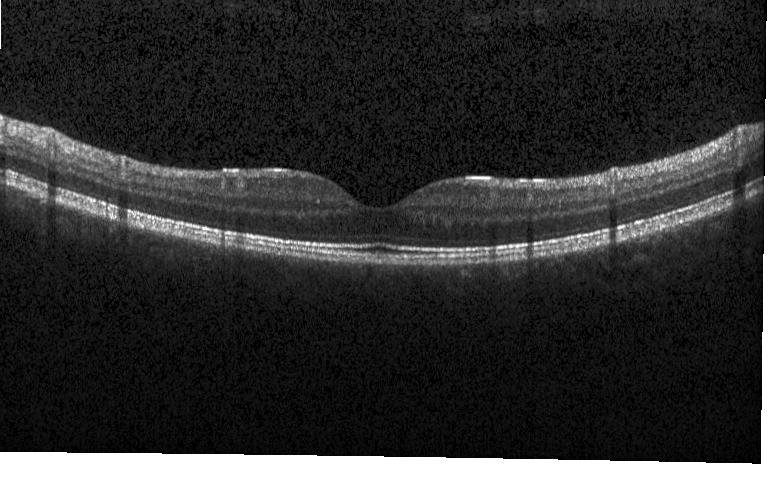
Optical coherence tomography B-scan. SD-OCT. Horizontal scan through the fovea. Assessment: no evidence of choroidal neovascularization, diabetic macular edema, or drusen.